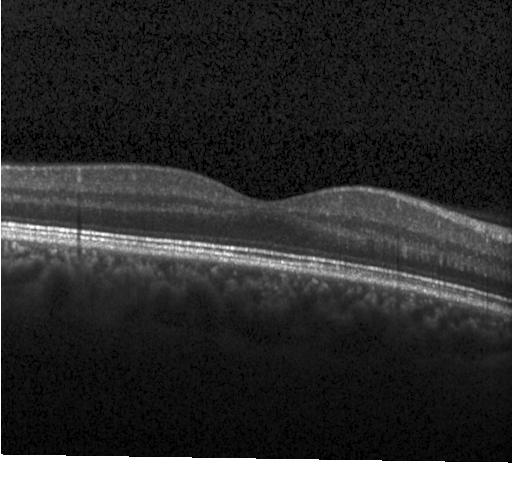 Spectral-domain OCT B-scan: no evidence of CNV, DME, or drusen.